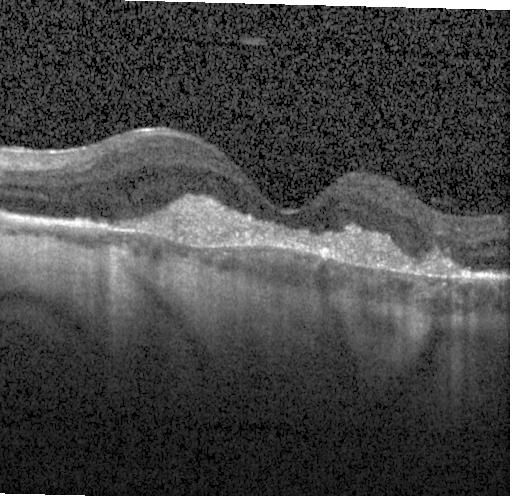
This B-scan demonstrates CNV.